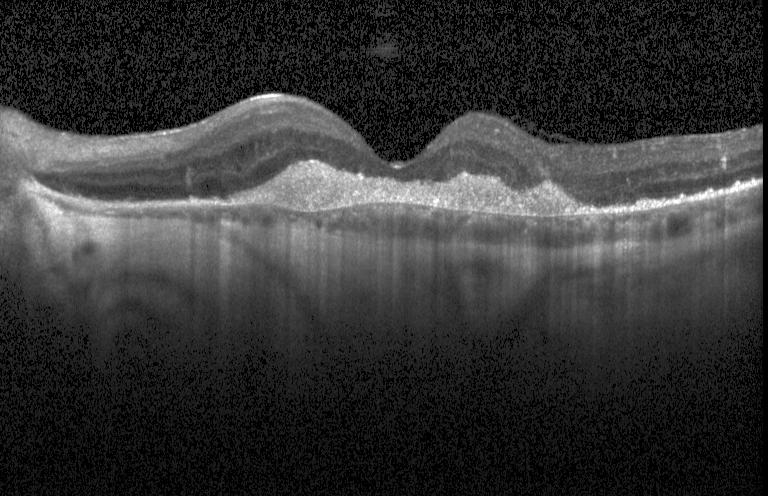

OCT line scan
This B-scan demonstrates a choroidal neovascular membrane.